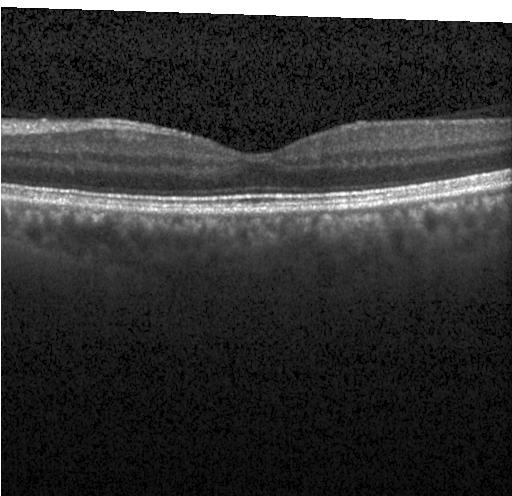

This B-scan demonstrates no evidence of choroidal neovascularization, diabetic macular edema, or drusen.